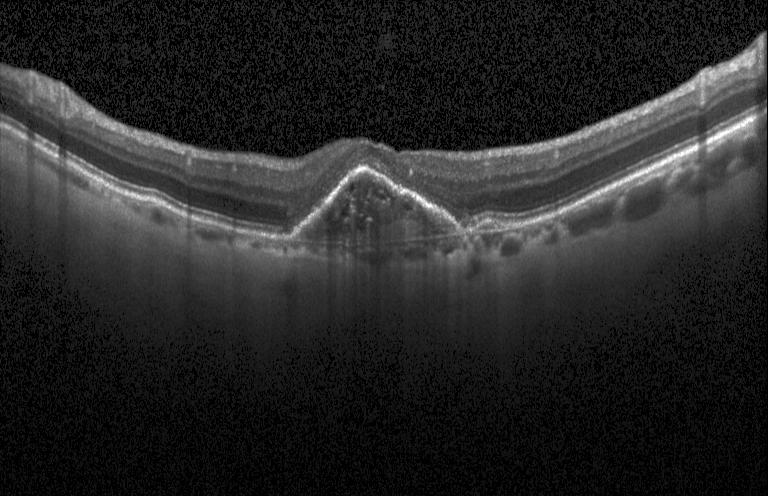
Impression: a choroidal neovascular membrane.